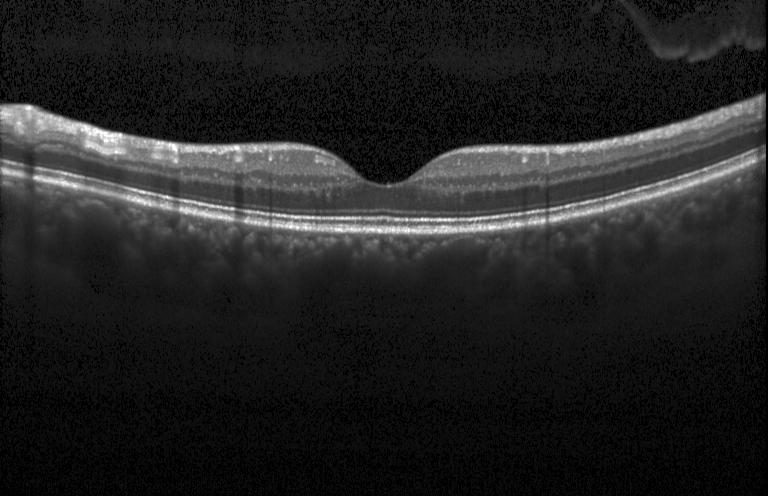

The scan shows no CNV, no DME, and no drusen.